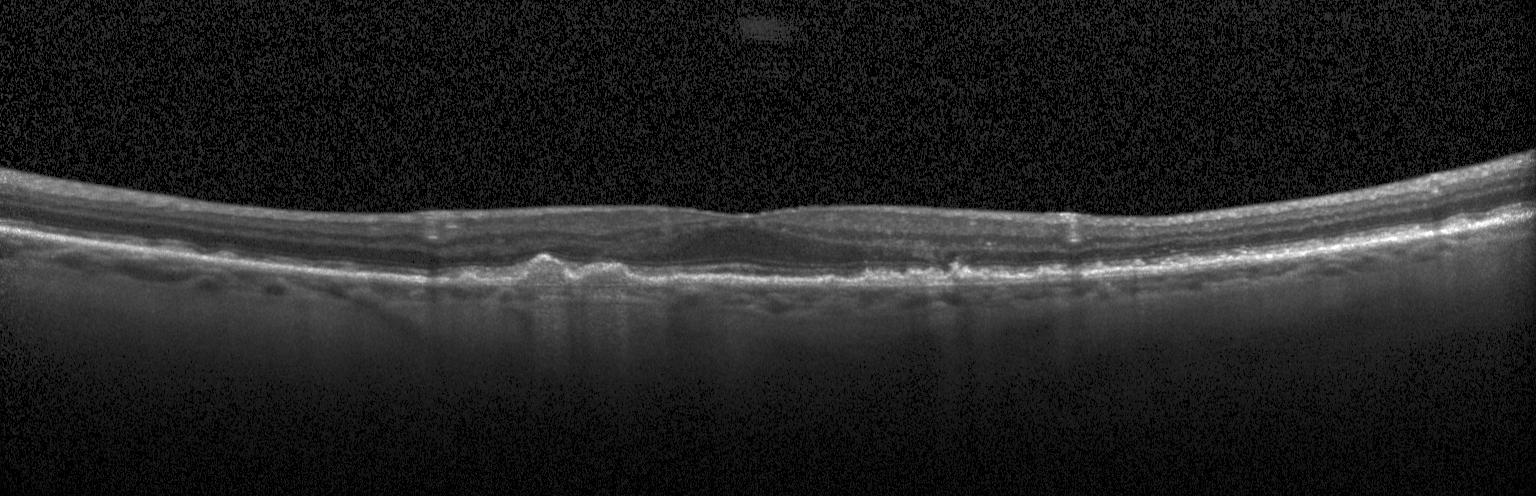 Horizontal scan through the fovea, optical coherence tomography B-scan — Finding: multiple drusen.